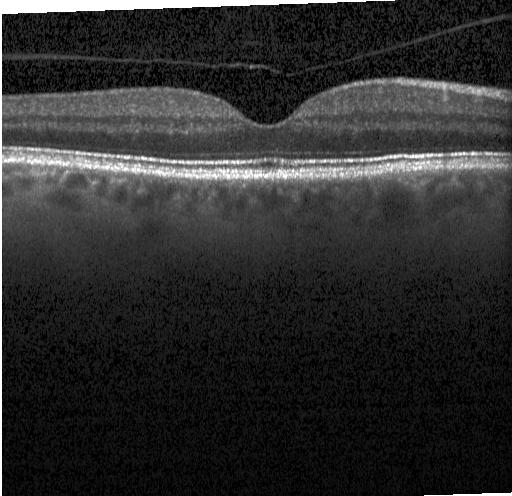

Optical coherence tomography B-scan. Acquired on a Heidelberg Spectralis. Diagnosis: no choroidal neovascularization, no diabetic macular edema, and no drusen.